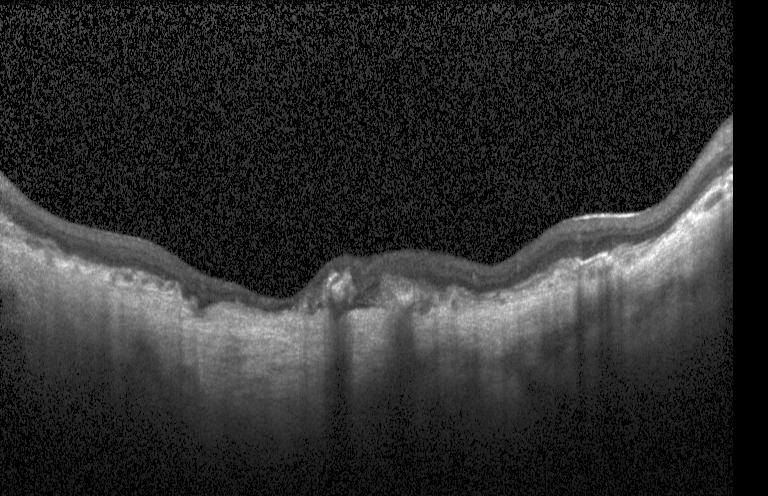

OCT B-scan. Horizontal scan through the fovea. Instrument: Heidelberg Spectralis
Diagnosis: a choroidal neovascular membrane.